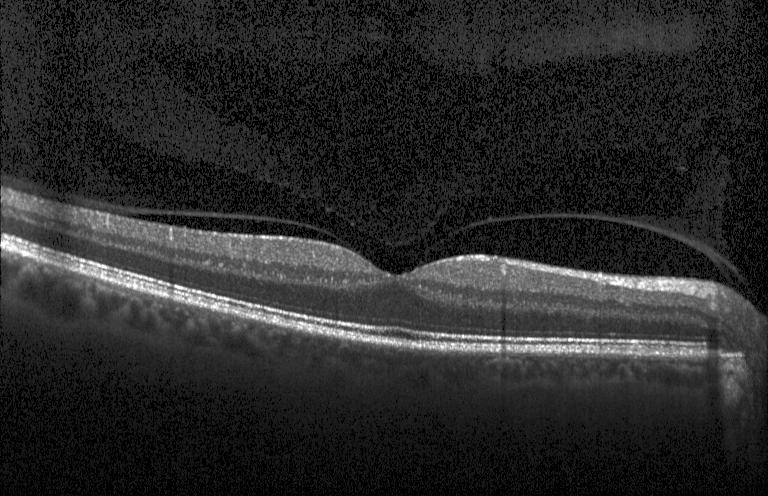
OCT B-scan.
Macular OCT: no evidence of choroidal neovascularization, diabetic macular edema, or drusen.